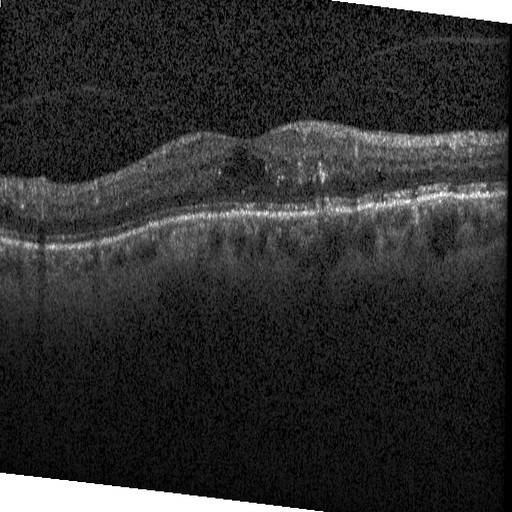
Retinal OCT cross-section. This B-scan demonstrates diabetic macular edema.